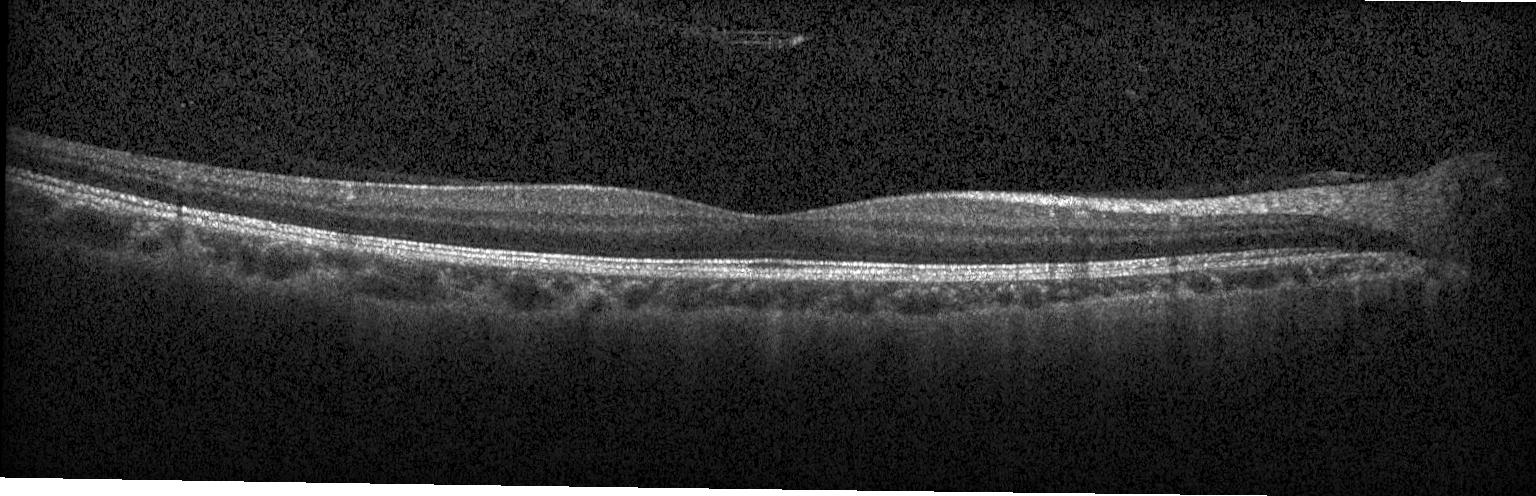 This B-scan demonstrates neither CNV, DME, nor drusen.